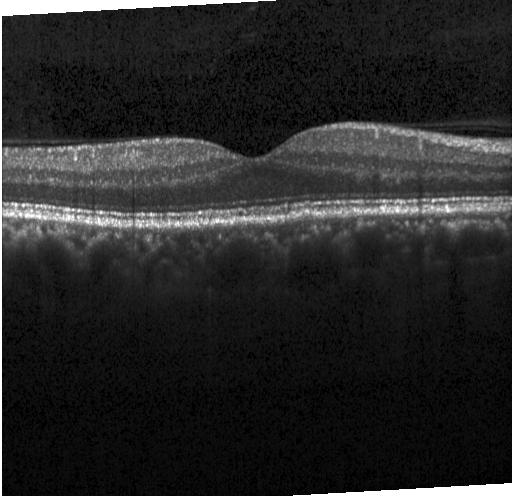 Impression: no evidence of choroidal neovascularization, diabetic macular edema, or drusen.